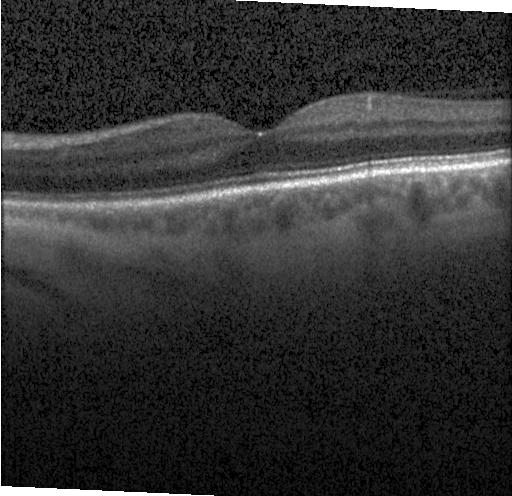

Macular scan. Optical coherence tomography B-scan — The scan shows no choroidal neovascularization, diabetic macular edema, or drusen.